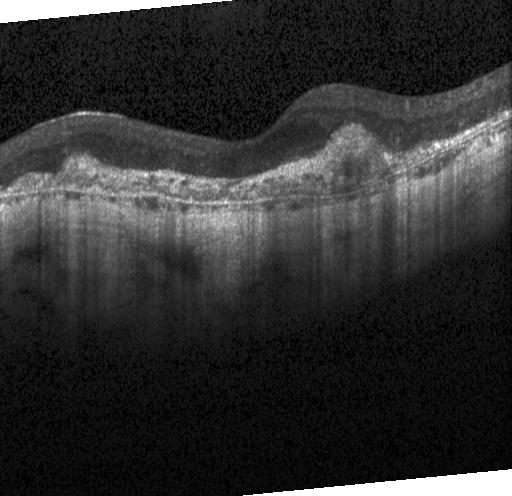 Assessment: a choroidal neovascular membrane.